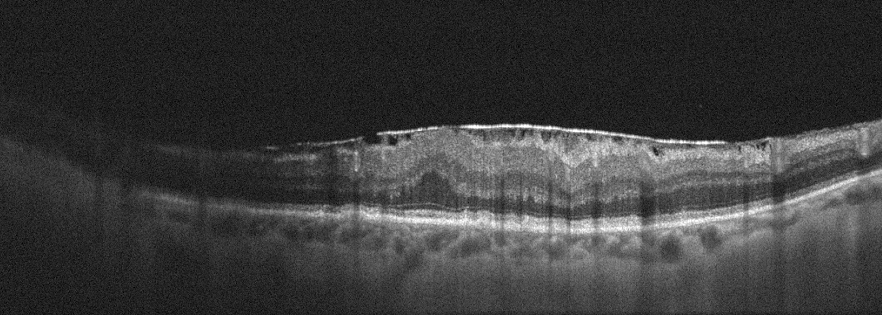
Right eye; retinal OCT B-scan; acquired on an Optovue Avanti RTVue XR
Dx: ERM.